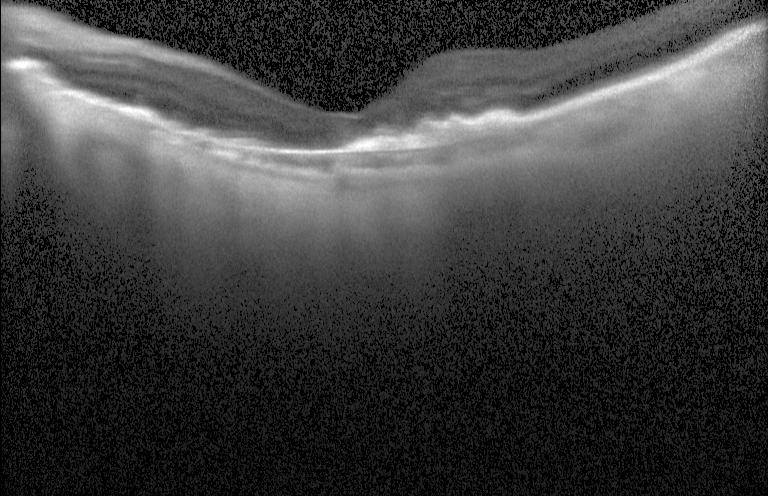

Retinal OCT cross-section. Heidelberg Spectralis. Impression: a choroidal neovascular membrane.